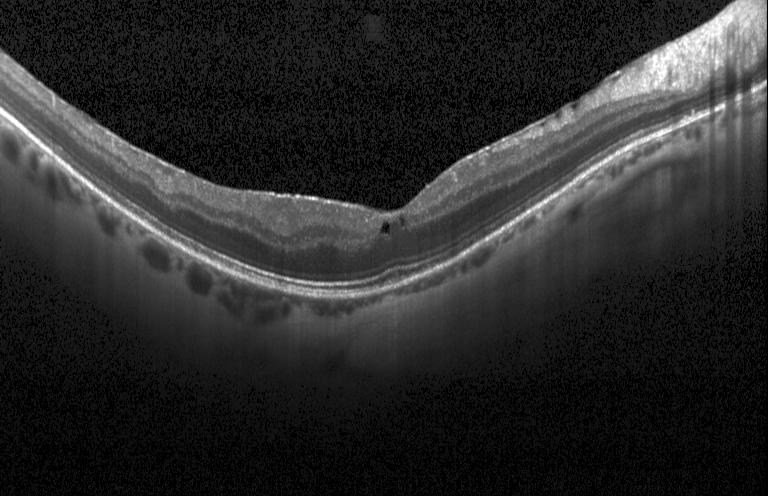

Optical coherence tomography B-scan. Diagnosis: DME.